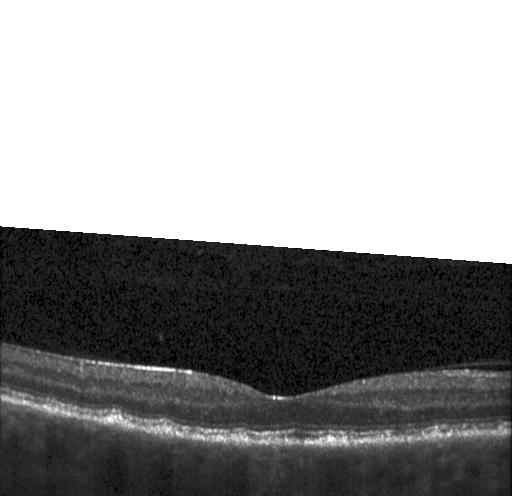 Macular OCT demonstrating drusen.